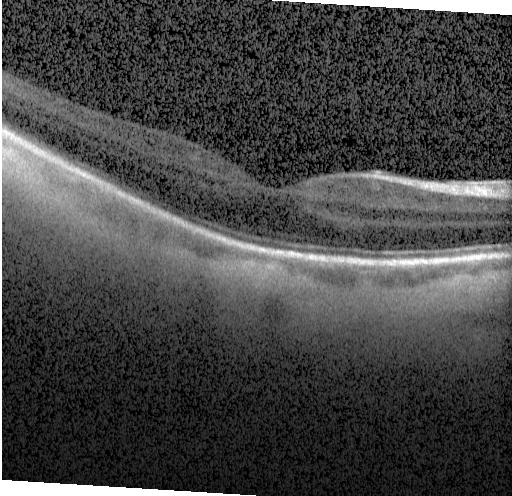

Retinal OCT cross-section — Finding: neither CNV, DME, nor drusen.